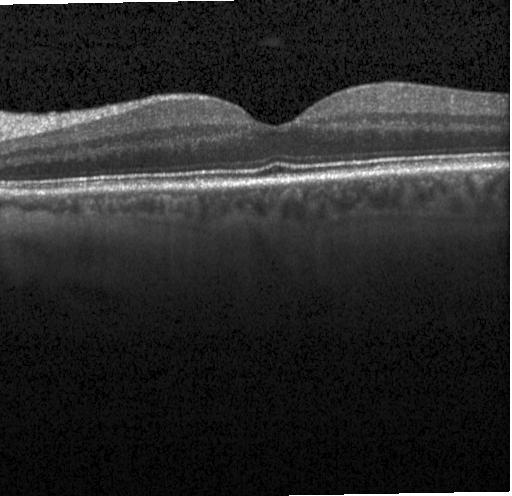

Heidelberg Spectralis OCT system. OCT B-scan. Horizontal scan through the fovea. SD-OCT
Dx: no choroidal neovascularization, diabetic macular edema, or drusen.